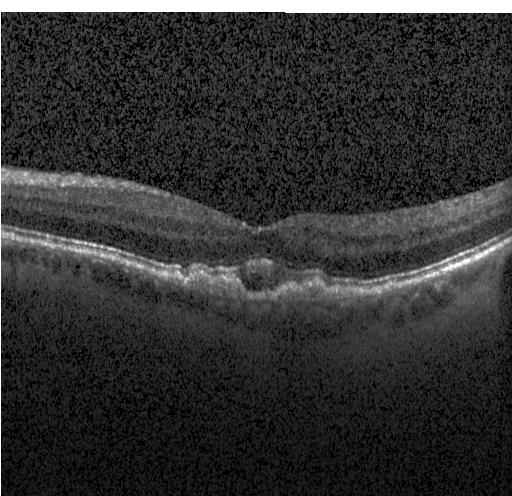
Heidelberg Spectralis OCT system · fovea-centered · retinal OCT B-scan. Multiple drusen.